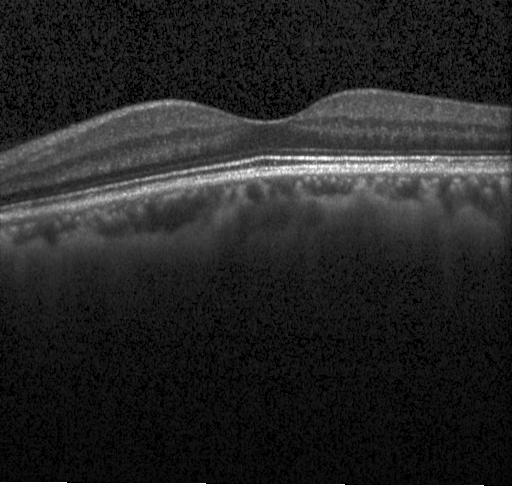

Retinal OCT cross-section showing no CNV, DME, or drusen.